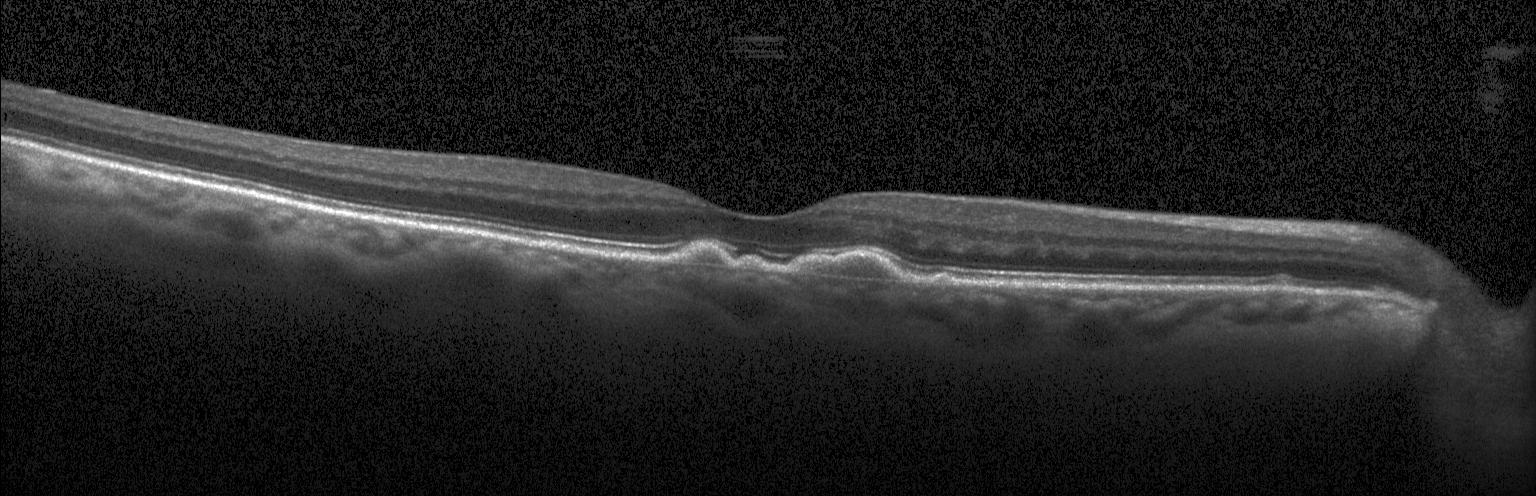
OCT B-scan; spectral-domain OCT.
Diagnosis: sub-RPE drusenoid deposits.